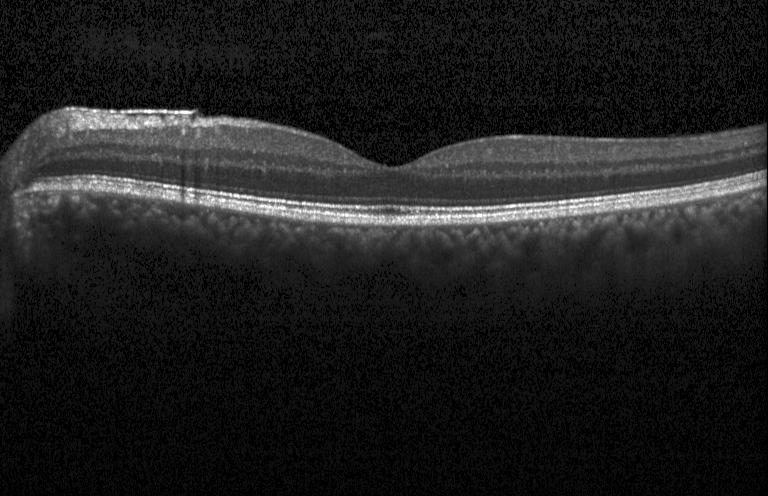 Macular OCT: neither CNV, DME, nor drusen.